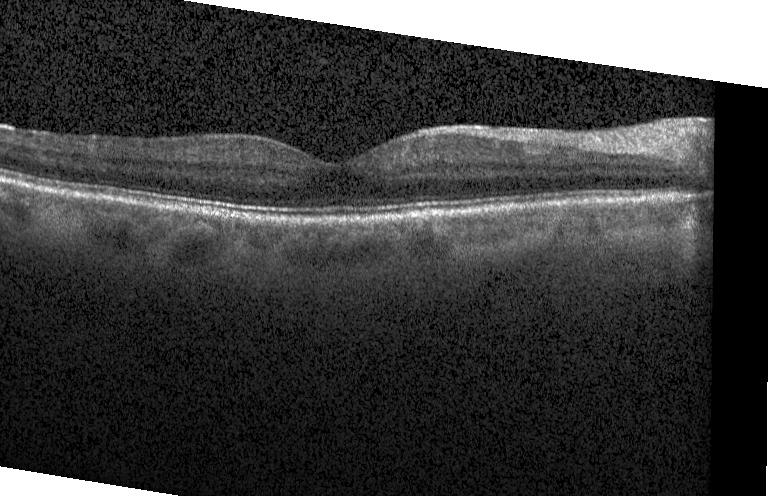

Instrument: Heidelberg Spectralis · optical coherence tomography scan · macular scan · spectral-domain optical coherence tomography — This B-scan demonstrates no CNV, no DME, and no drusen.